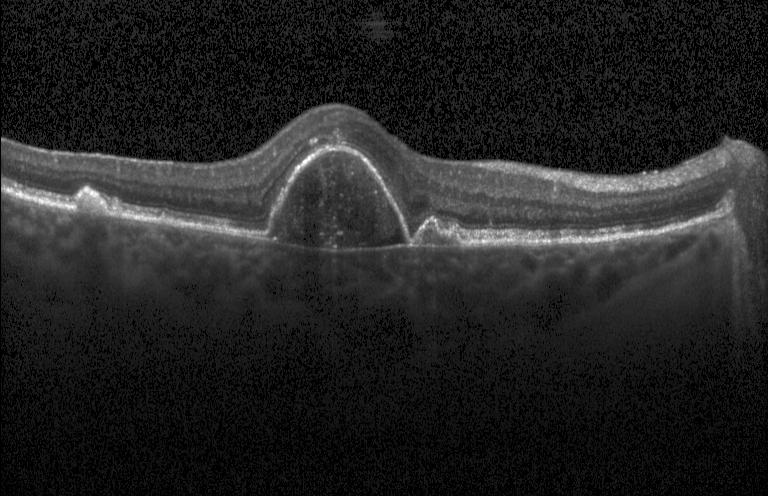
Macular OCT: a choroidal neovascular membrane.